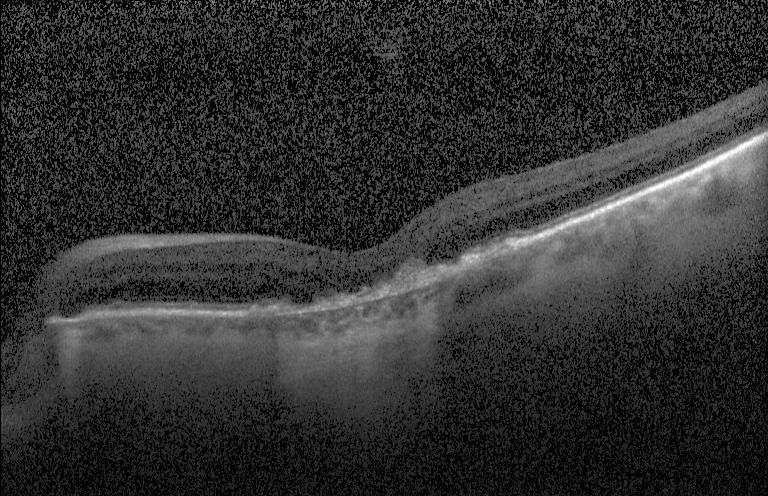

The scan shows a choroidal neovascular membrane.